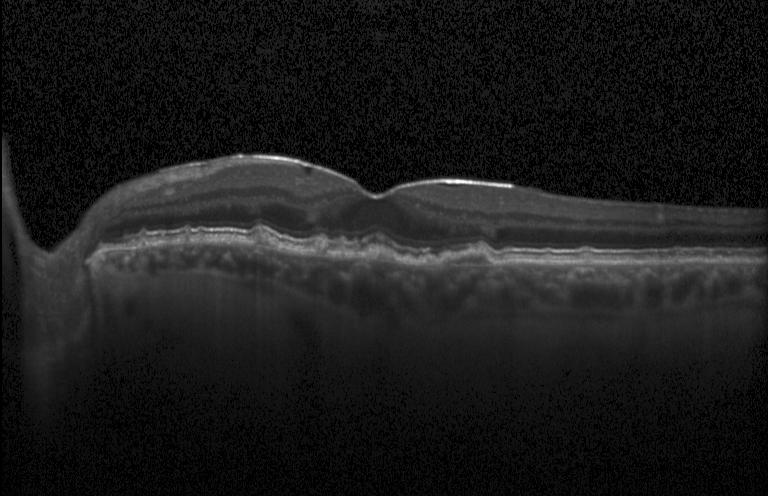
OCT B-scan. Instrument: Heidelberg Spectralis — Impression: sub-RPE drusenoid deposits.